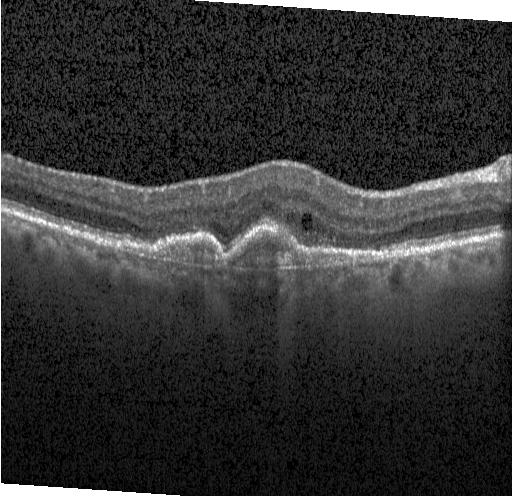

Macular OCT demonstrating choroidal neovascularization (CNV).